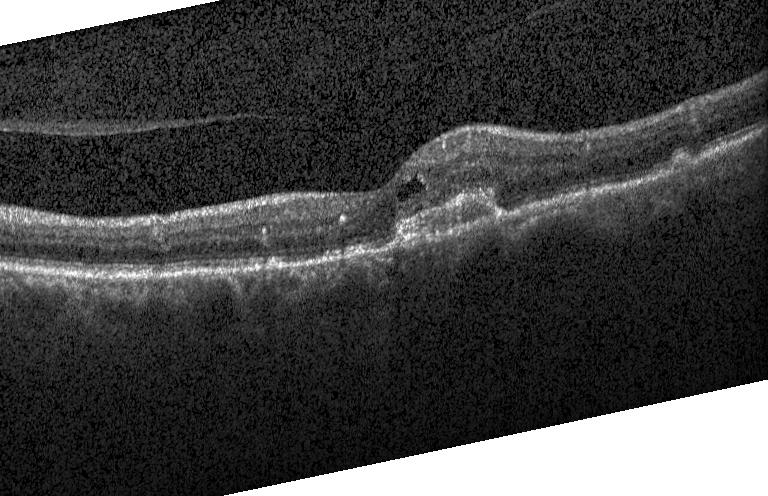

Horizontal scan through the fovea. Optical coherence tomography B-scan. SD-OCT
OCT finding: CNV.